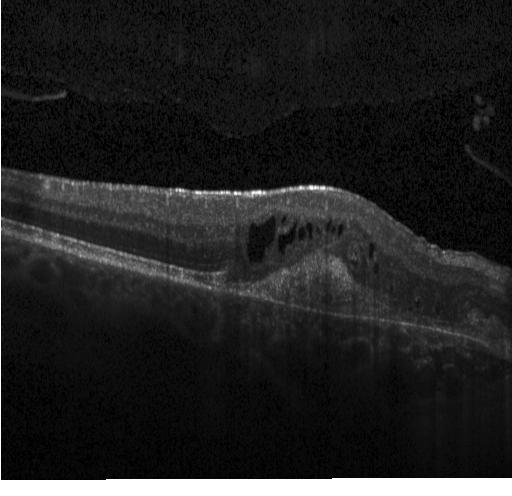
Centered on the fovea, OCT B-scan
Impression: a choroidal neovascular membrane.